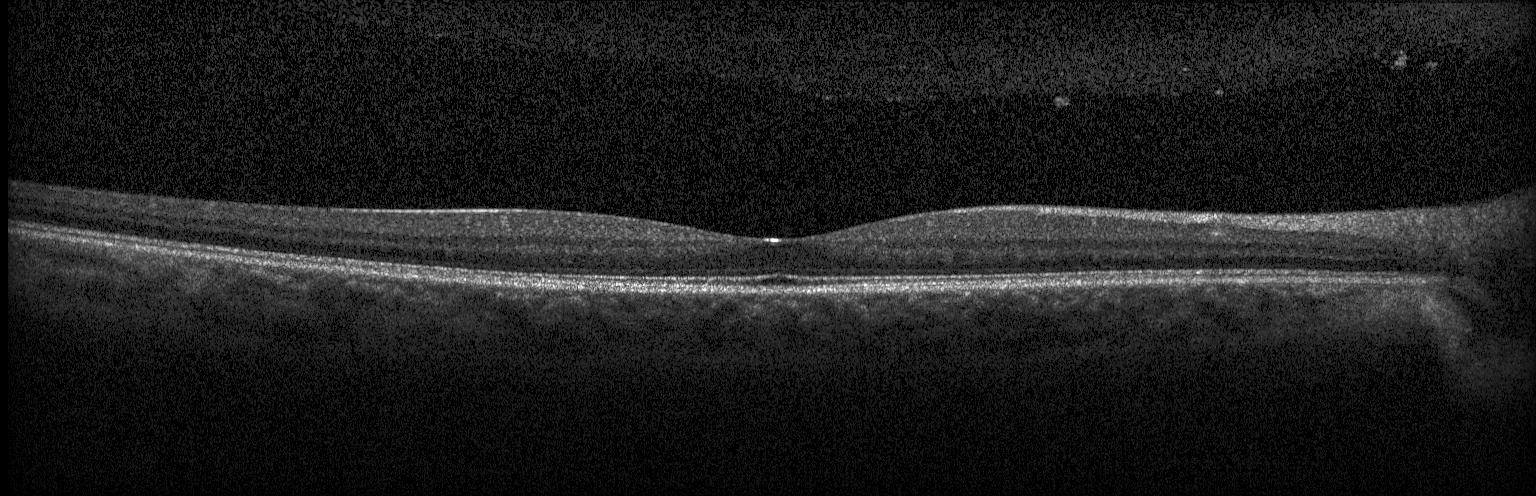 Optical coherence tomography B-scan
No choroidal neovascularization, diabetic macular edema, or drusen.